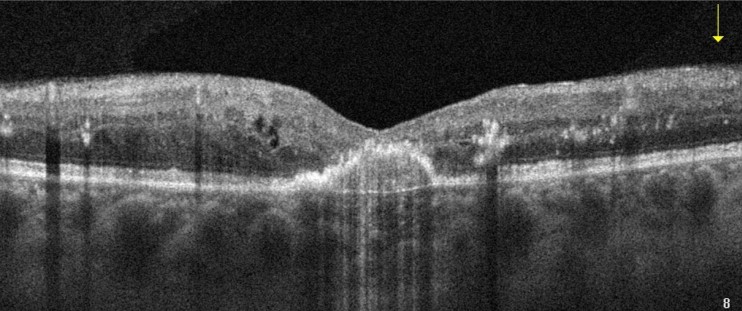 This B-scan demonstrates DME.